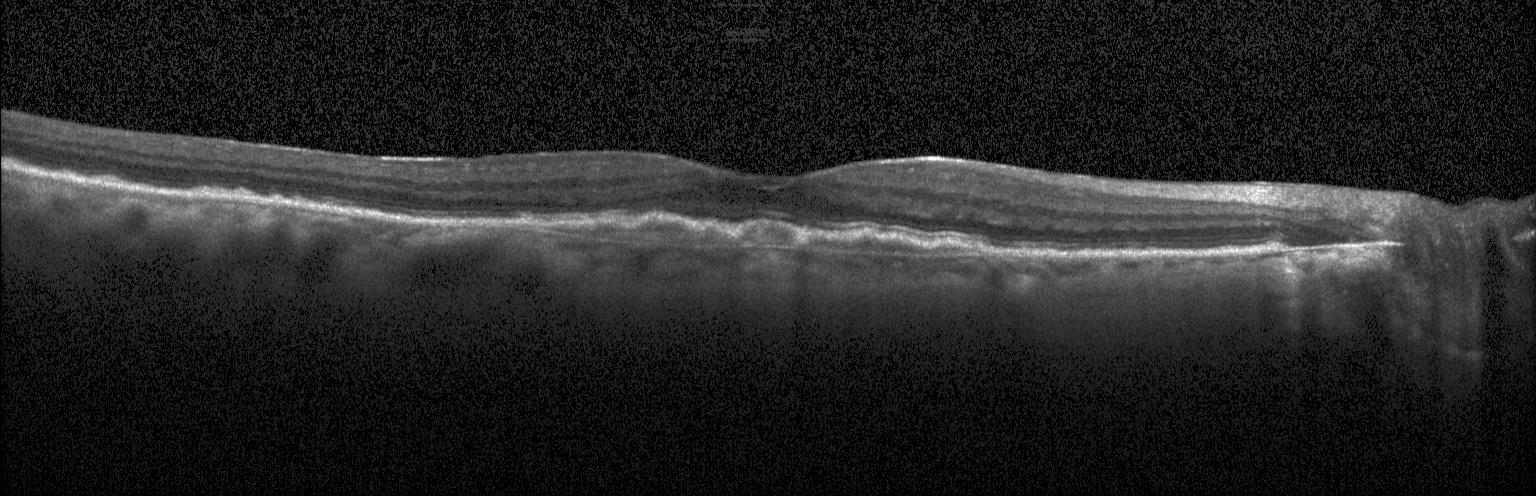
Heidelberg Spectralis OCT system. Retinal OCT B-scan — Diagnosis: choroidal neovascularization.